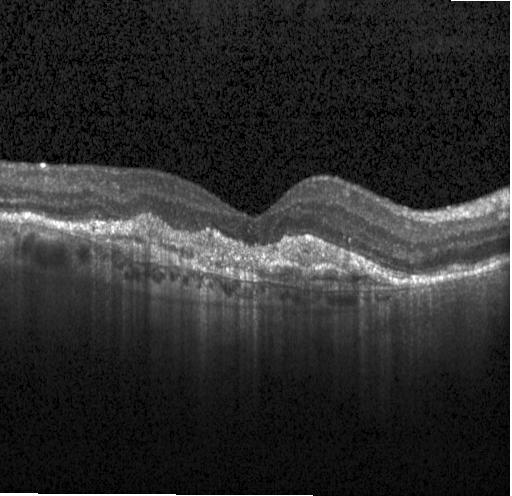
Spectral-domain optical coherence tomography. Optical coherence tomography B-scan
Diagnosis: CNV.